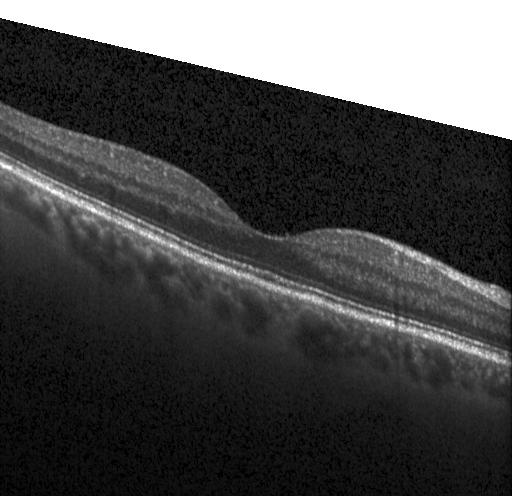
SD-OCT. Retinal OCT B-scan — Macular OCT: neither choroidal neovascularization, diabetic macular edema, nor drusen.